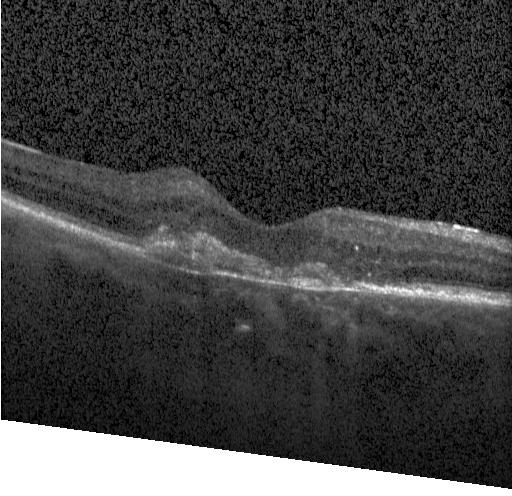

Spectral-domain optical coherence tomography, retinal OCT cross-section, Heidelberg Spectralis
Finding: a choroidal neovascular membrane.